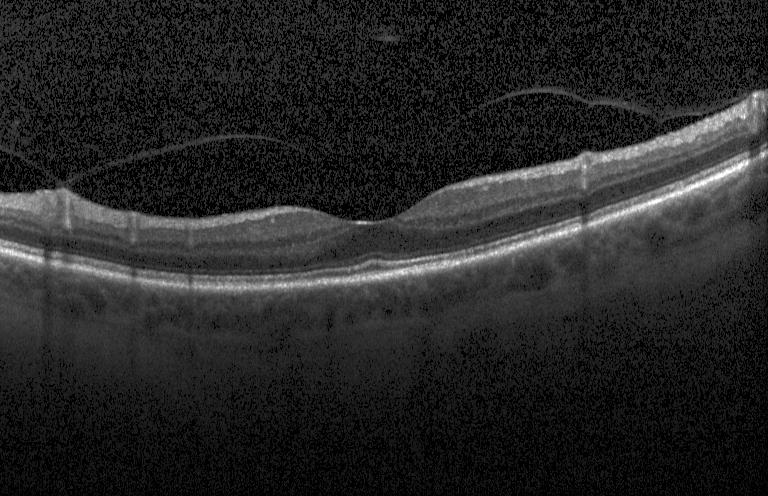
Spectral-domain optical coherence tomography; optical coherence tomography scan; macular scan; Heidelberg Spectralis OCT system.
Diagnosis: no CNV, DME, or drusen.